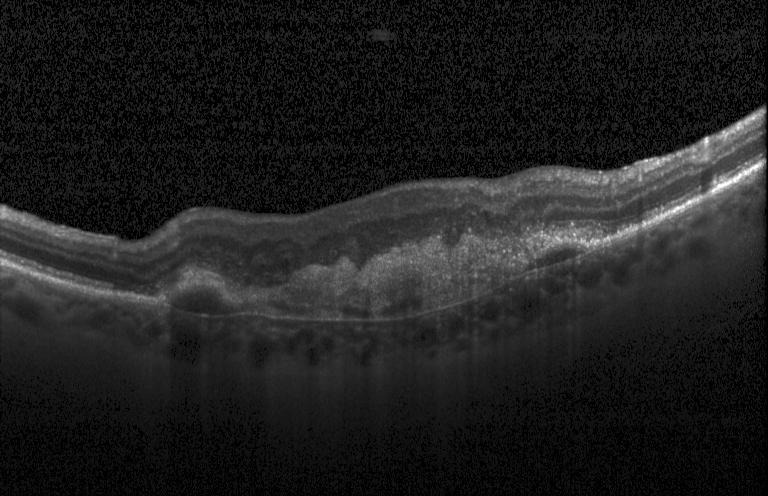
Optical coherence tomography B-scan. Macular scan
Dx: a choroidal neovascular membrane.